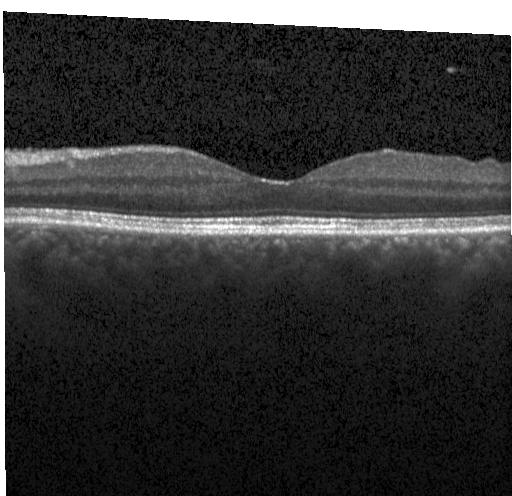

Retinal OCT cross-section
Diagnosis: neither choroidal neovascularization, diabetic macular edema, nor drusen.